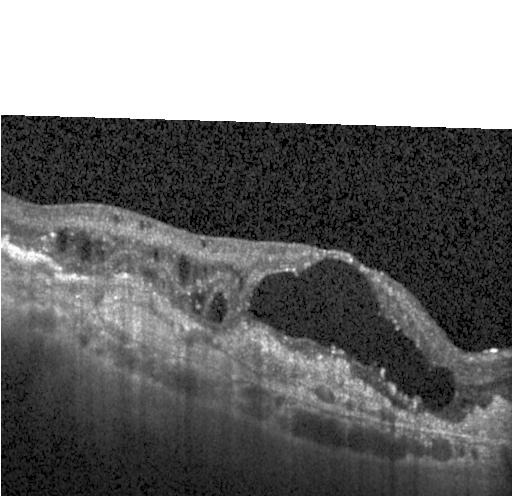
Spectral-domain OCT B-scan: a choroidal neovascular membrane.